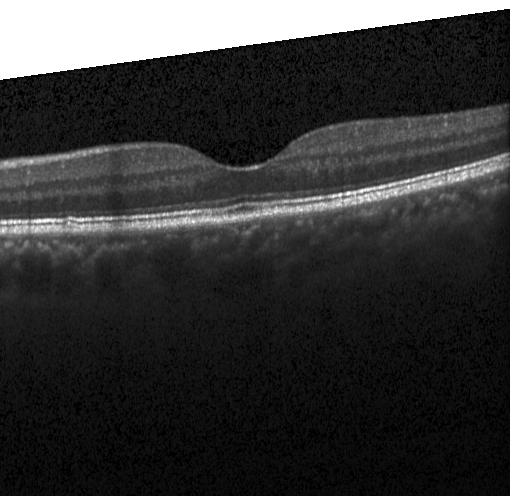 Retinal OCT B-scan · Heidelberg Spectralis · through the macula.
Macular OCT: neither choroidal neovascularization, diabetic macular edema, nor drusen.